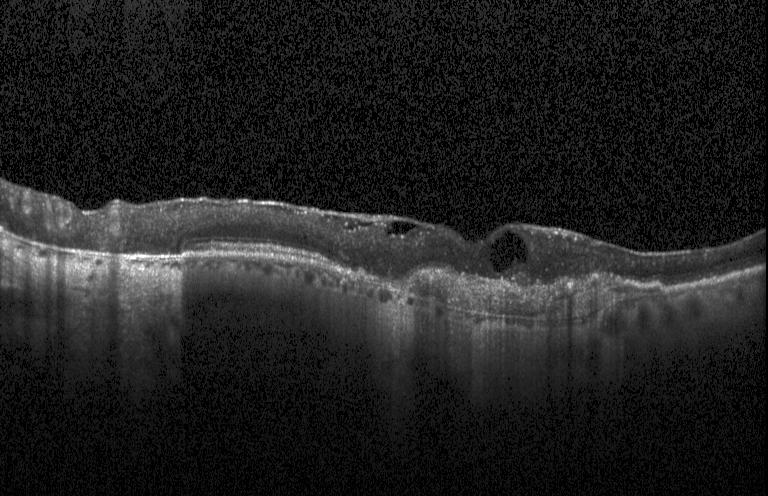
Heidelberg Spectralis OCT system; spectral-domain OCT; optical coherence tomography B-scan; macular scan
Impression: CNV.